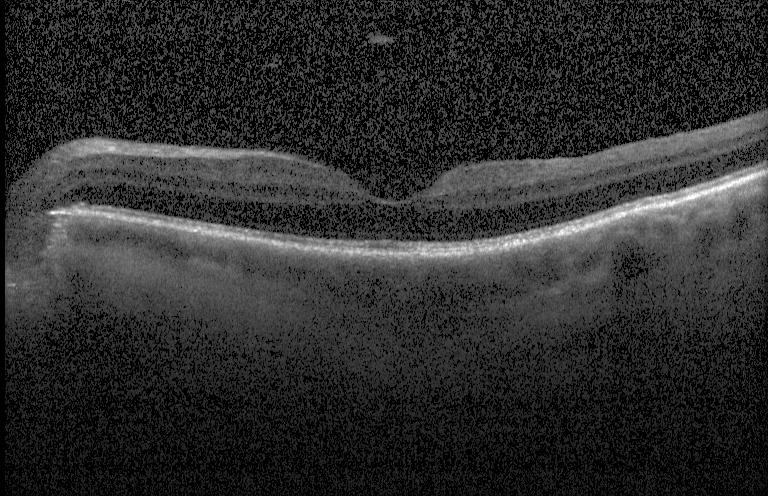
No choroidal neovascularization, no diabetic macular edema, and no drusen.